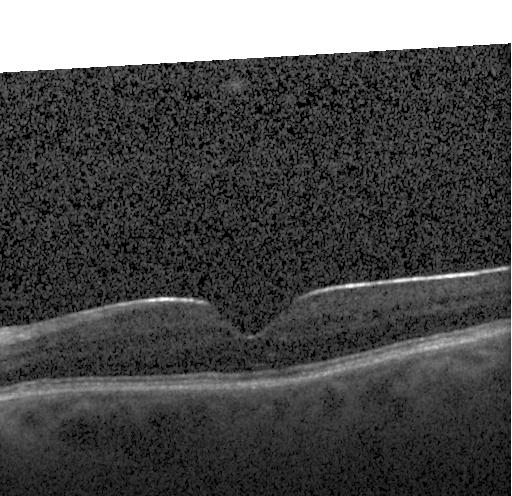
Through the macula; instrument: Heidelberg Spectralis; spectral-domain OCT; optical coherence tomography B-scan.
This B-scan demonstrates no CNV, DME, or drusen.